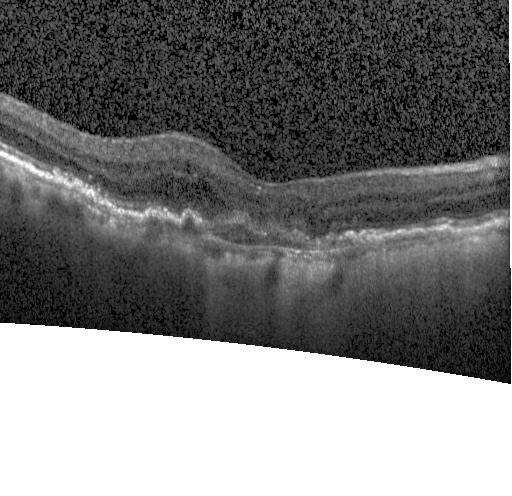
OCT line scan.
The scan shows a choroidal neovascular membrane.